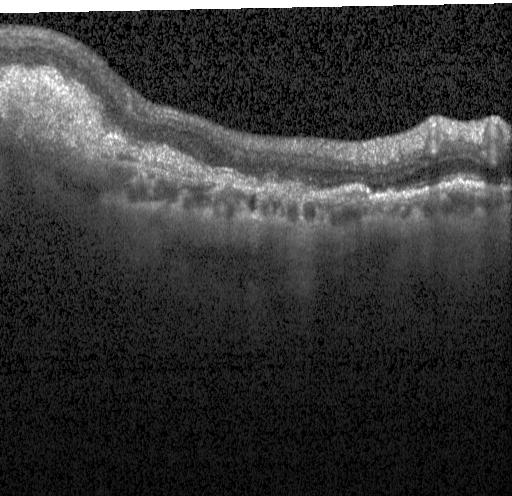
Spectral-domain OCT, OCT B-scan, acquired on a Heidelberg Spectralis — Impression: choroidal neovascularization.